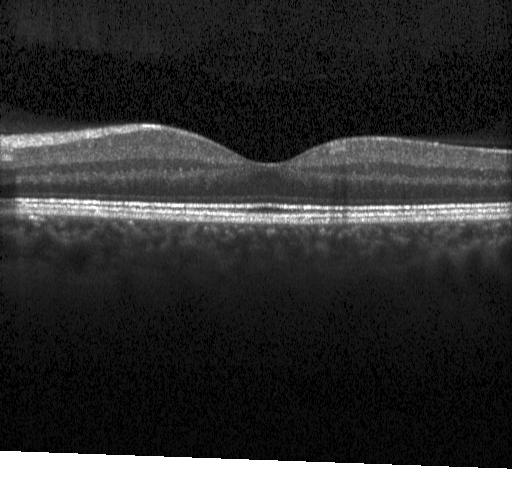
Retinal OCT cross-section showing neither choroidal neovascularization, diabetic macular edema, nor drusen.